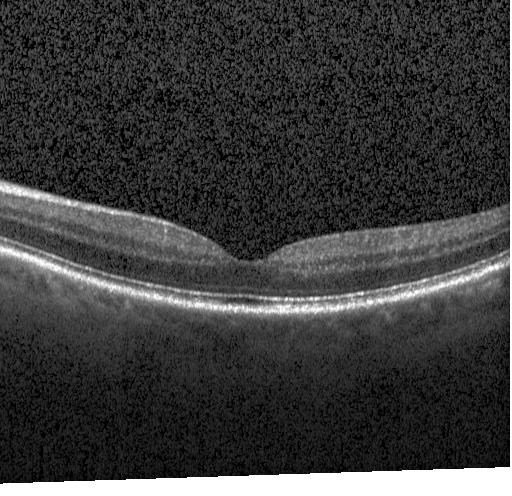

Macular OCT: no evidence of choroidal neovascularization, diabetic macular edema, or drusen.